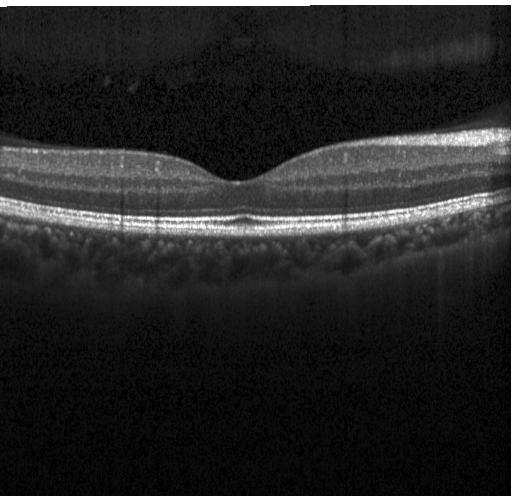

Optical coherence tomography B-scan.
OCT finding: no choroidal neovascularization, diabetic macular edema, or drusen.